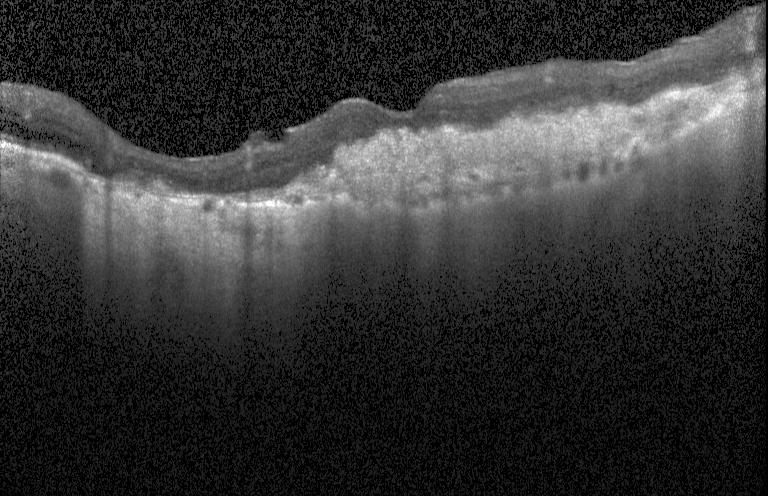
Diagnosis: choroidal neovascularization.